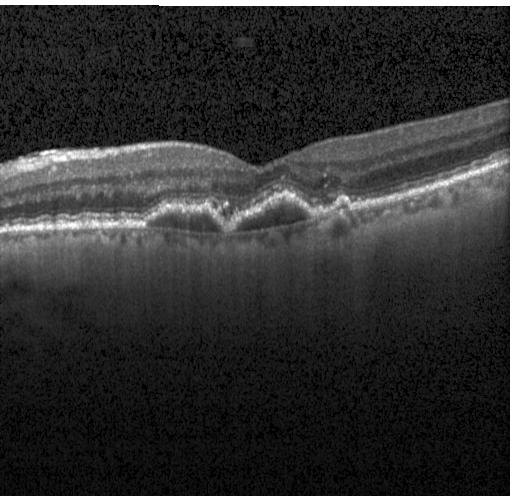
OCT B-scan, Heidelberg Spectralis. Assessment: a choroidal neovascular membrane.